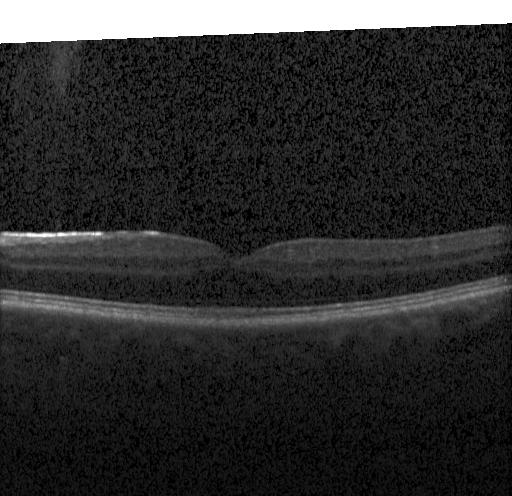
Heidelberg Spectralis; retinal OCT B-scan; macular scan; SD-OCT.
The scan shows no choroidal neovascularization, no diabetic macular edema, and no drusen.